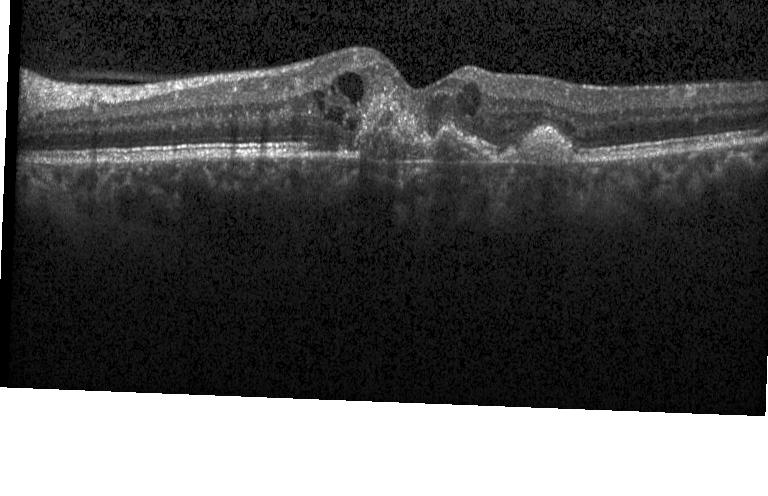 The scan shows choroidal neovascularization (CNV).